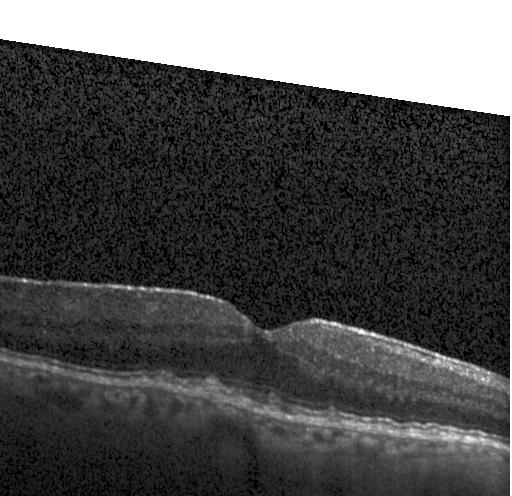 Macular OCT: sub-RPE drusenoid deposits.